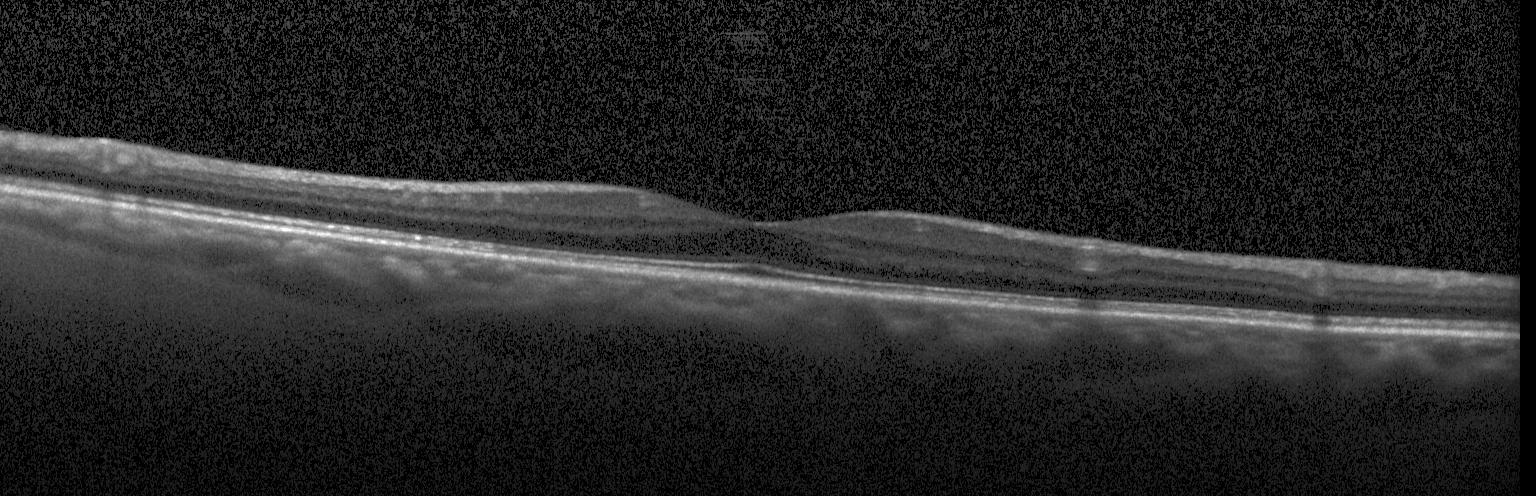 OCT line scan.
Assessment: no choroidal neovascularization, diabetic macular edema, or drusen.